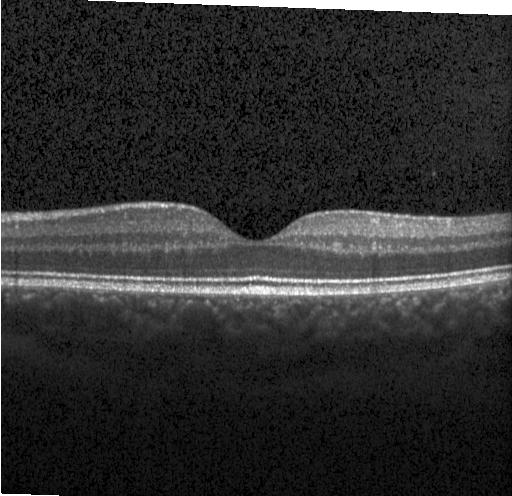
Through the macula; spectral-domain optical coherence tomography; optical coherence tomography B-scan
Finding: no evidence of CNV, DME, or drusen.